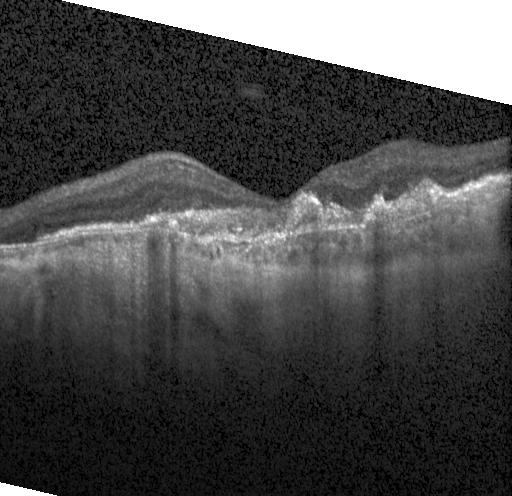
Impression: choroidal neovascularization.